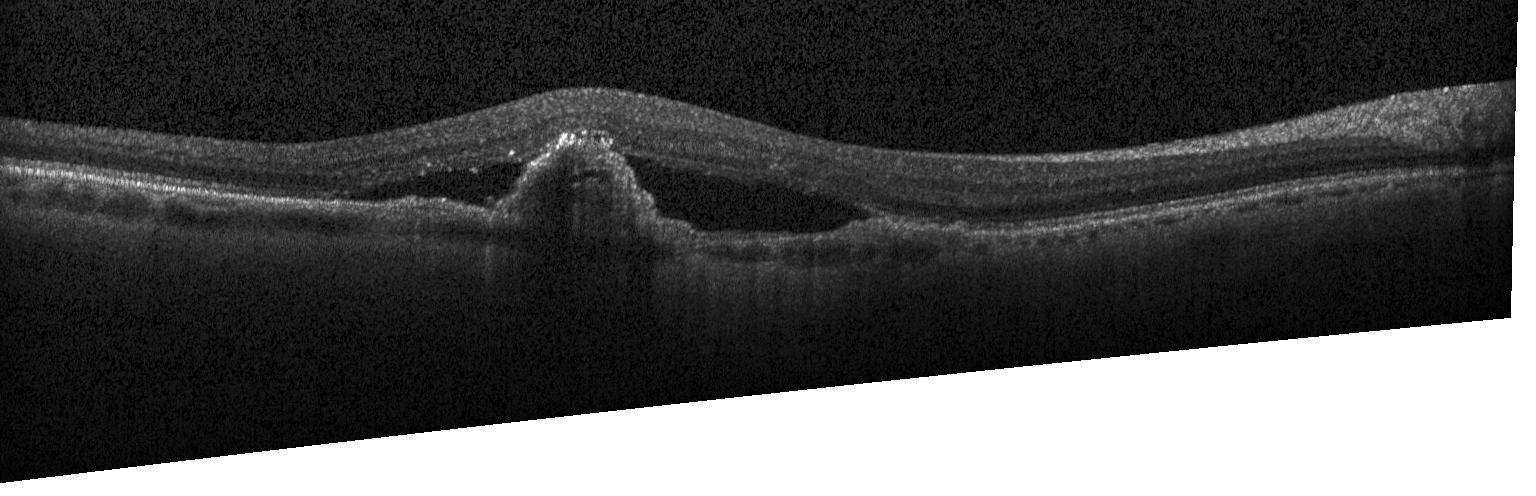

Diagnosis: CNV.